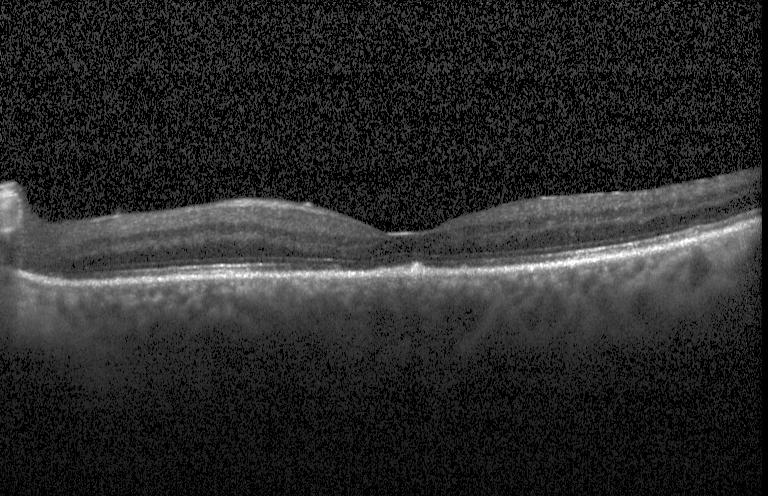

OCT finding: multiple drusen.